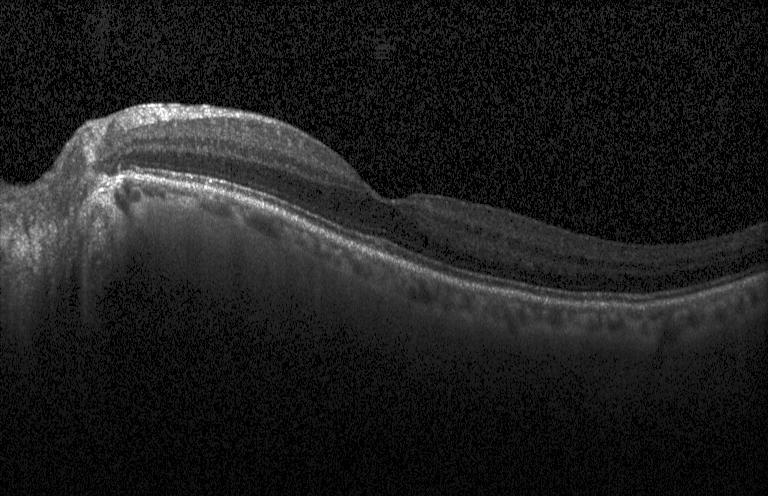 This B-scan demonstrates no evidence of CNV, DME, or drusen.